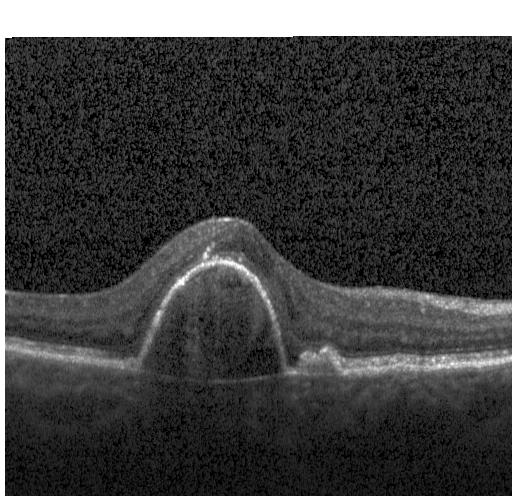

Spectral-domain optical coherence tomography, instrument: Heidelberg Spectralis, OCT line scan. Dx: choroidal neovascularization (CNV).